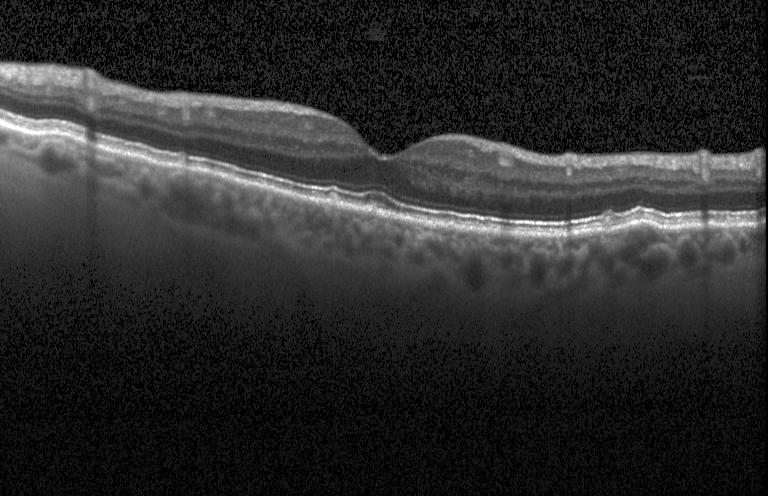 Optical coherence tomography B-scan. Assessment: multiple drusen.